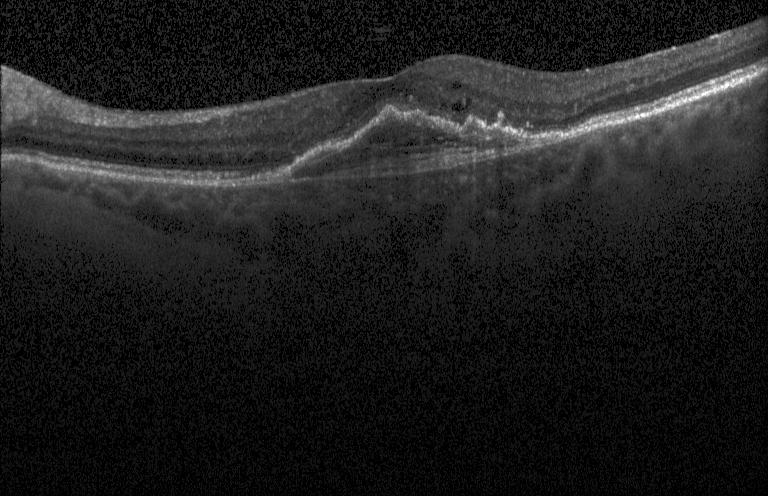

Optical coherence tomography scan — This B-scan demonstrates a choroidal neovascular membrane.